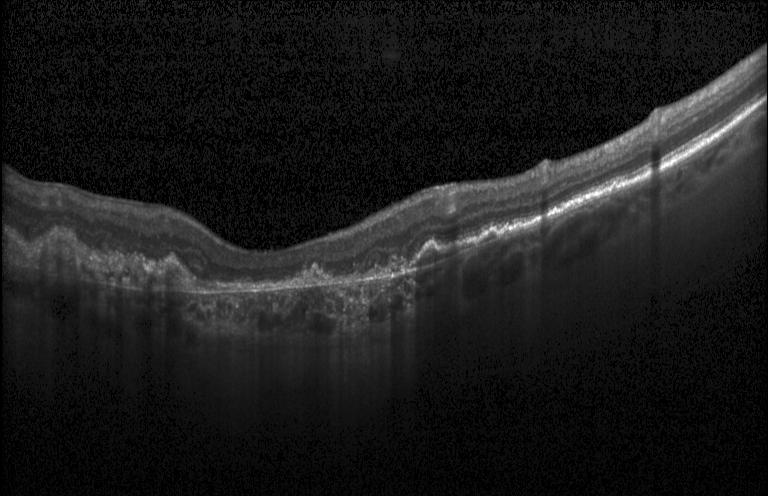

Heidelberg Spectralis OCT system, OCT line scan. Choroidal neovascularization.